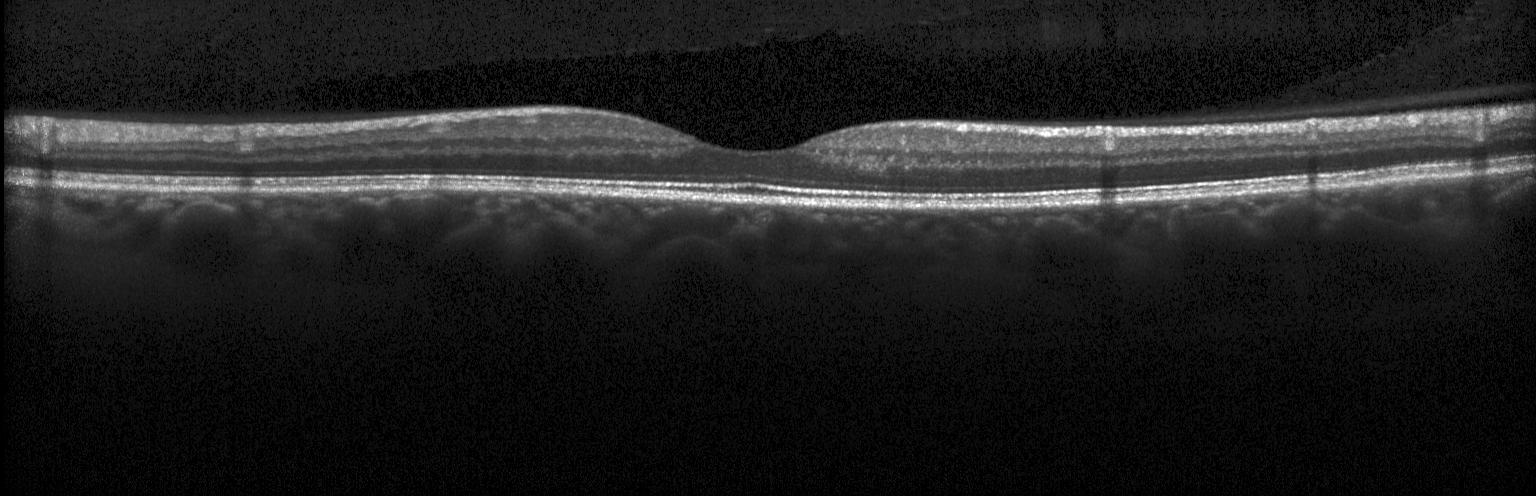
OCT B-scan; SD-OCT — Impression: no CNV, no DME, and no drusen.